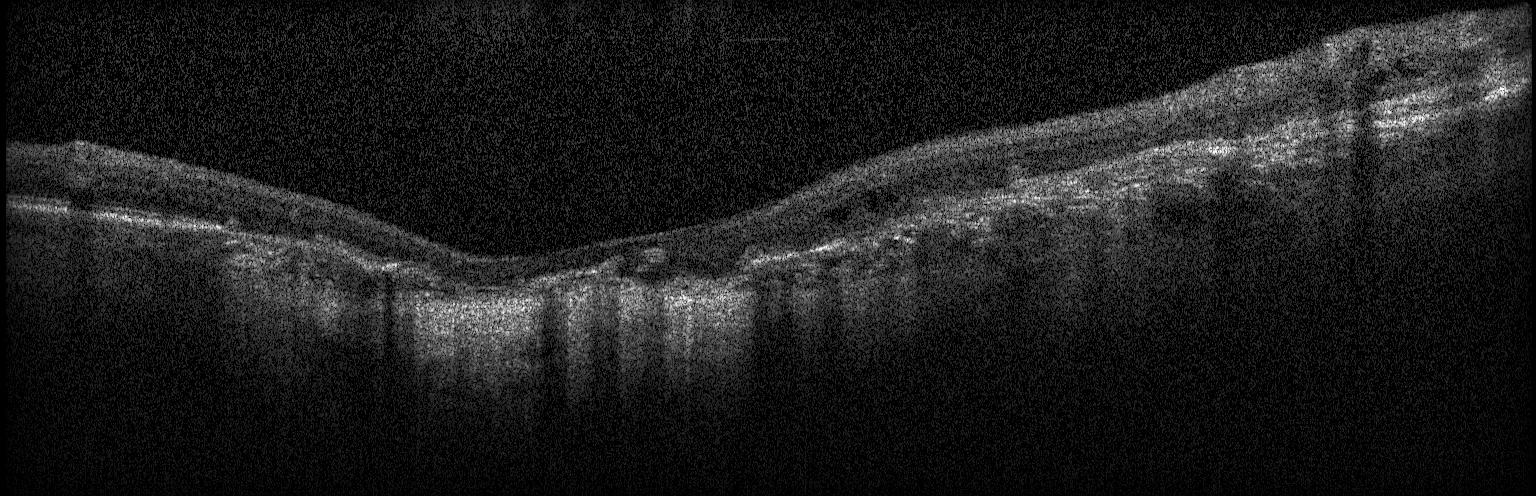

OCT line scan. Dx: CNV.